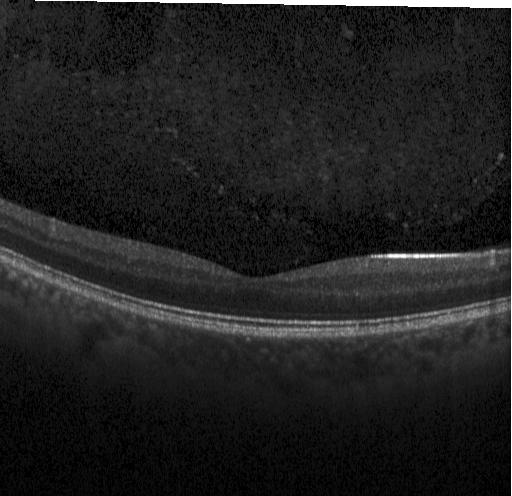 Retinal OCT cross-section.
Finding: no evidence of choroidal neovascularization, diabetic macular edema, or drusen.